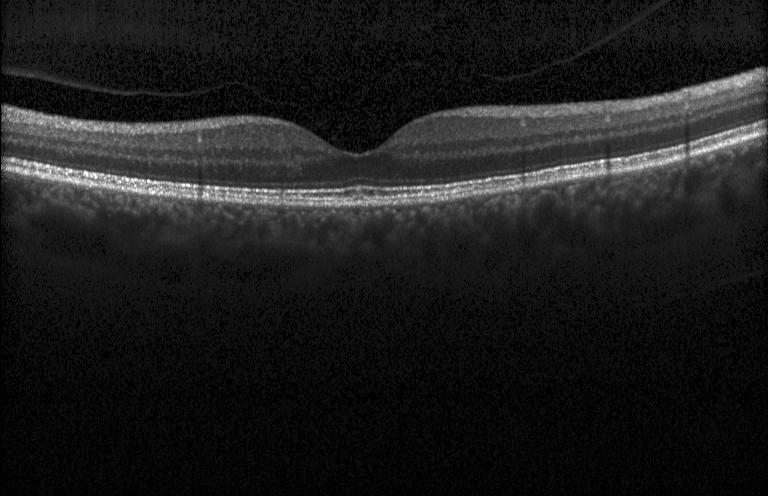

Optical coherence tomography B-scan · SD-OCT · Heidelberg Spectralis OCT system · centered on the fovea — This B-scan demonstrates no evidence of CNV, DME, or drusen.